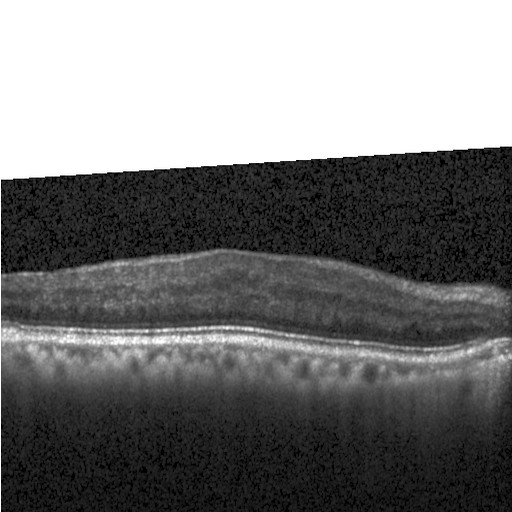 Instrument: Heidelberg Spectralis; SD-OCT; optical coherence tomography B-scan; fovea-centered.
Finding: DME.